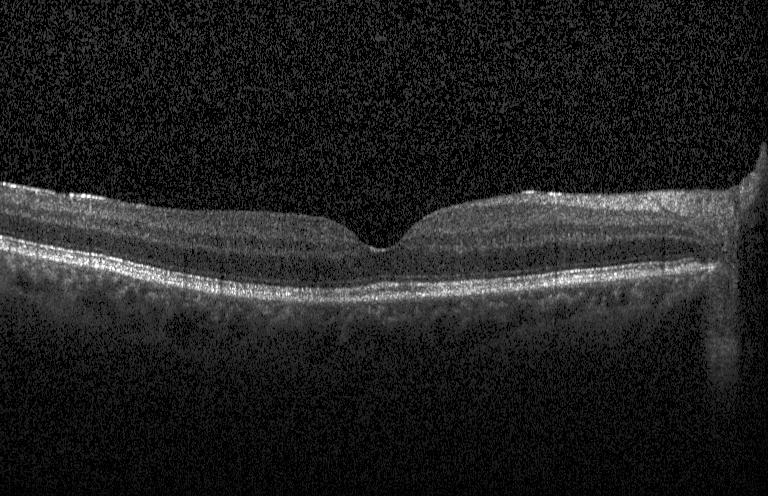

Finding: no evidence of CNV, DME, or drusen.